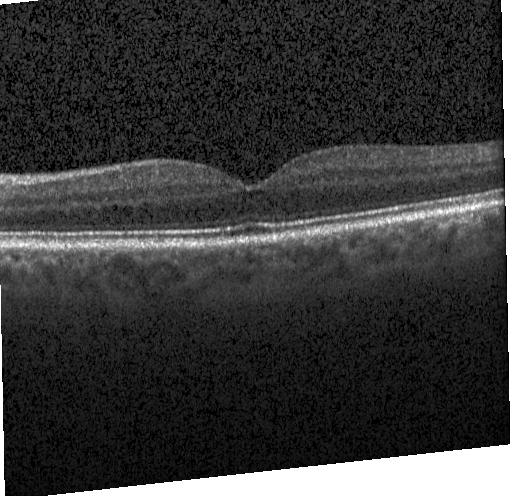
OCT line scan.
Finding: neither CNV, DME, nor drusen.